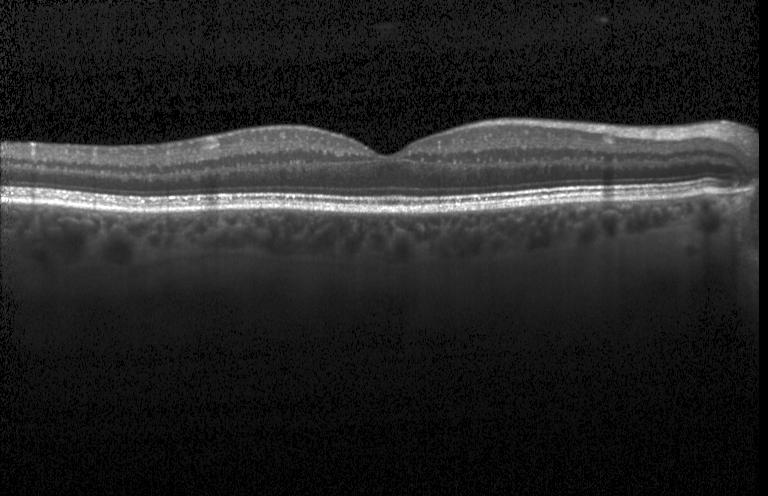

Spectral-domain OCT. Optical coherence tomography scan. Heidelberg Spectralis OCT system — Finding: neither choroidal neovascularization, diabetic macular edema, nor drusen.